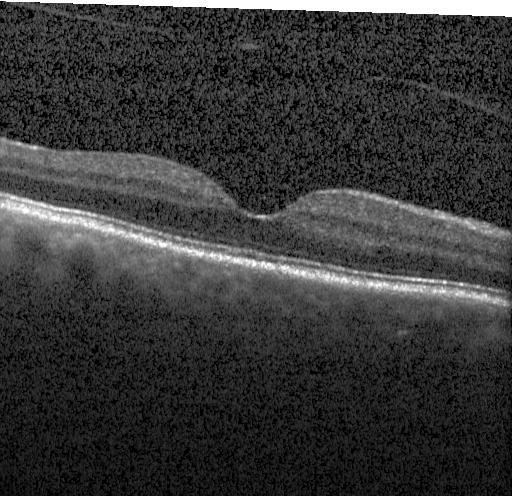
Centered on the fovea. Optical coherence tomography scan. SD-OCT — Finding: neither choroidal neovascularization, diabetic macular edema, nor drusen.